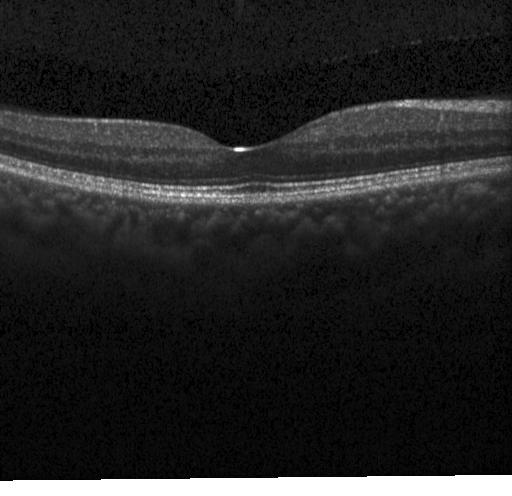

Fovea-centered; OCT line scan; instrument: Heidelberg Spectralis; spectral-domain OCT. Macular OCT: no evidence of CNV, DME, or drusen.